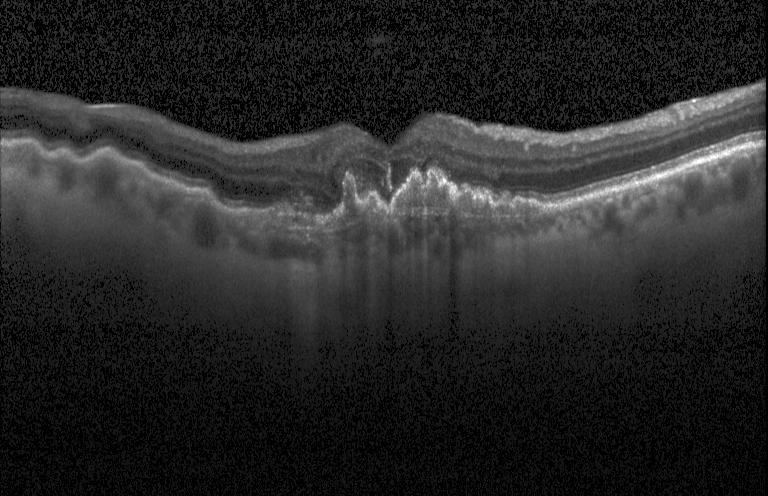
Choroidal neovascularization (CNV).